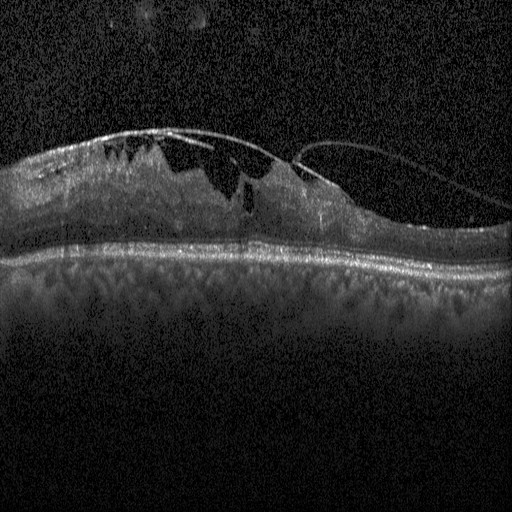 Macular OCT: DME.